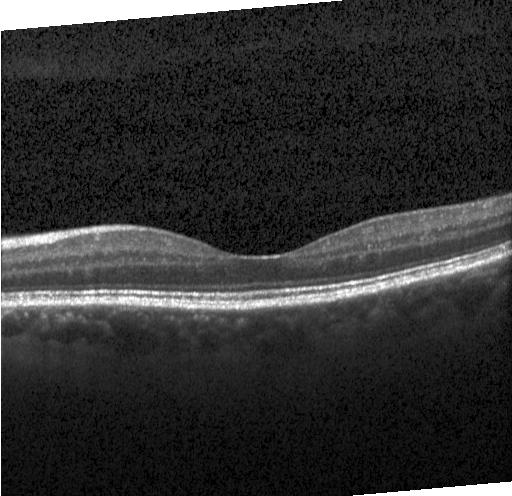
The scan shows no evidence of CNV, DME, or drusen.